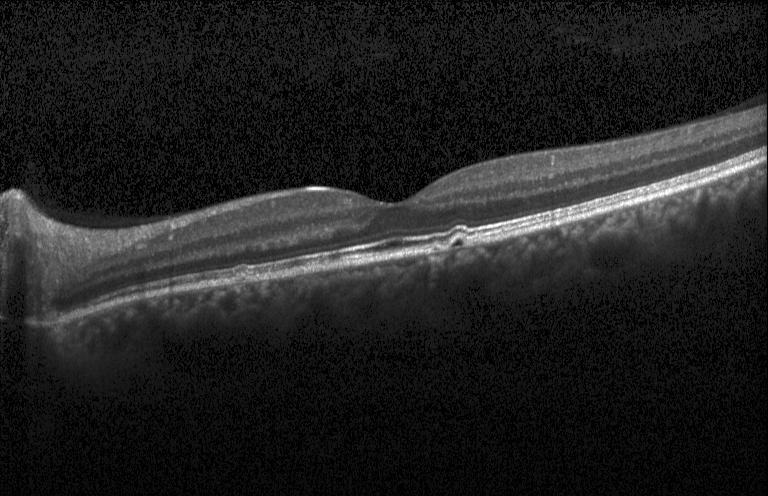
Optical coherence tomography scan · macular scan — The scan shows sub-RPE drusenoid deposits.